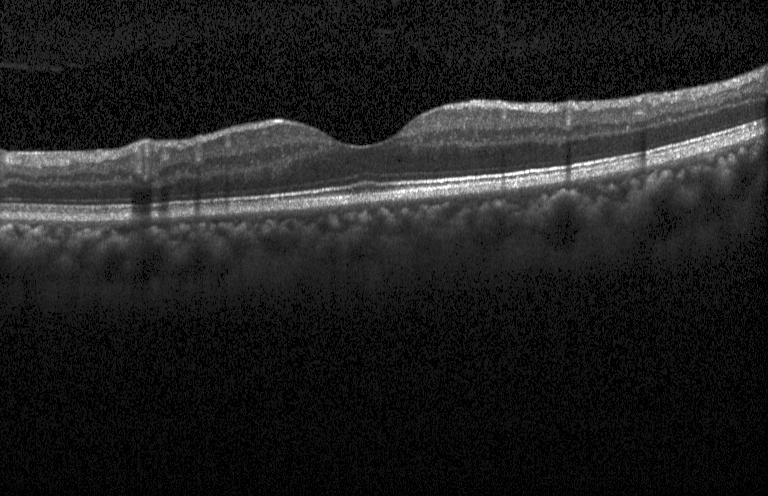
Finding: no choroidal neovascularization, no diabetic macular edema, and no drusen.